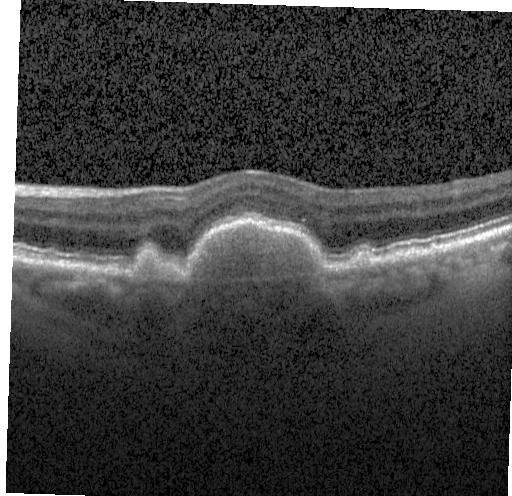 Macular OCT demonstrating CNV.